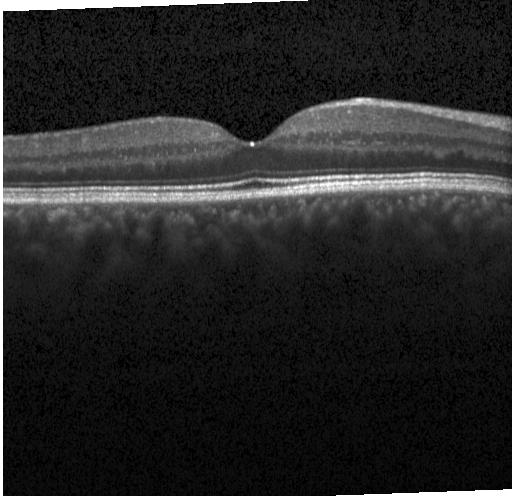

OCT finding: no CNV, DME, or drusen.